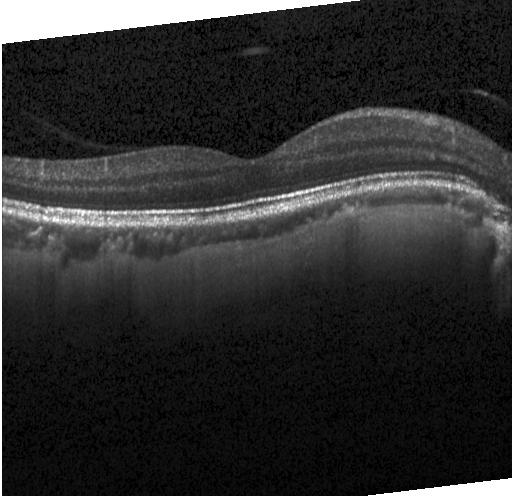

OCT line scan · macular scan.
The scan shows no CNV, no DME, and no drusen.